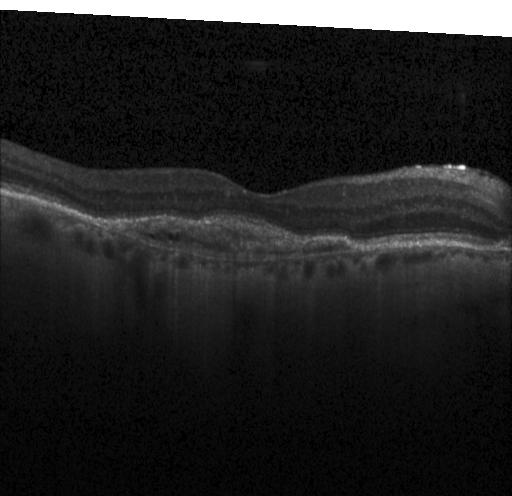
SD-OCT, retinal OCT B-scan.
Impression: a choroidal neovascular membrane.